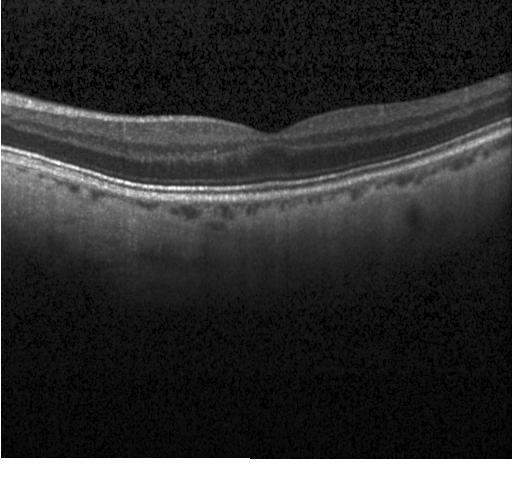 No CNV, no DME, and no drusen.